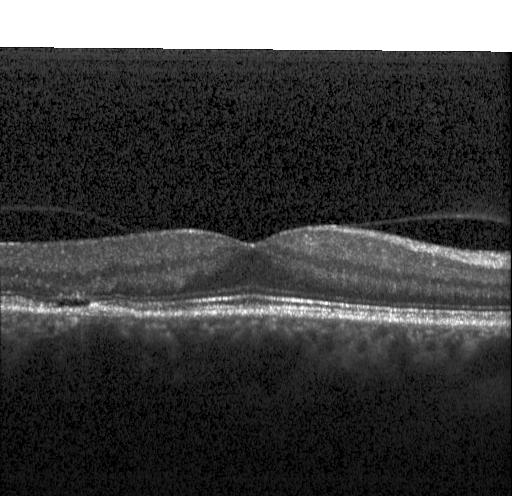
Spectral-domain optical coherence tomography, Heidelberg Spectralis OCT system, horizontal scan through the fovea, optical coherence tomography scan
Macular OCT: a choroidal neovascular membrane.